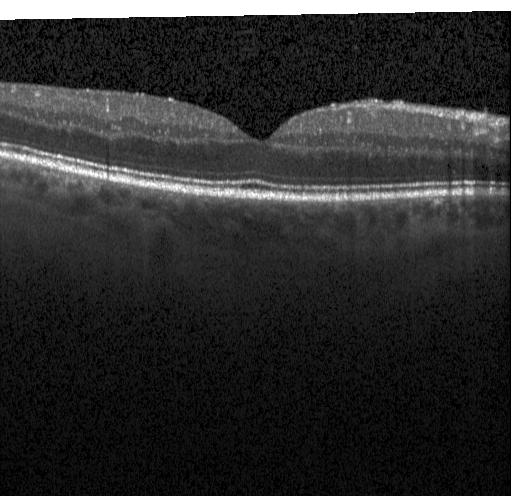 Spectral-domain OCT B-scan: no choroidal neovascularization, diabetic macular edema, or drusen.